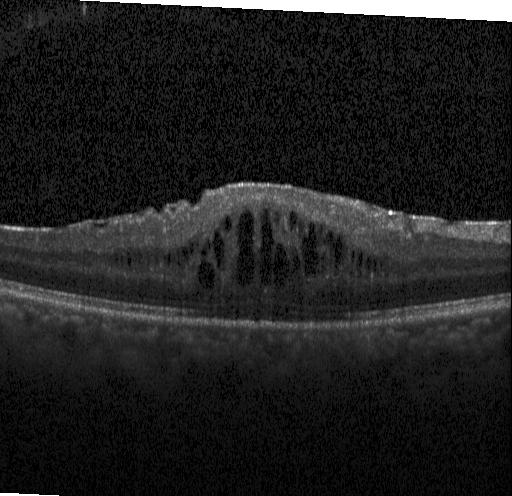
Spectral-domain optical coherence tomography. Centered on the fovea. Heidelberg Spectralis. OCT line scan — Macular OCT: DME.